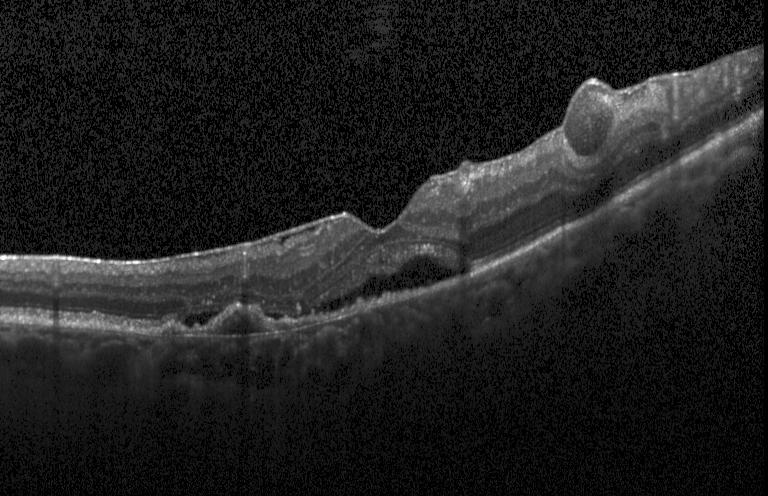
Instrument: Heidelberg Spectralis. Retinal OCT cross-section.
Finding: a choroidal neovascular membrane.